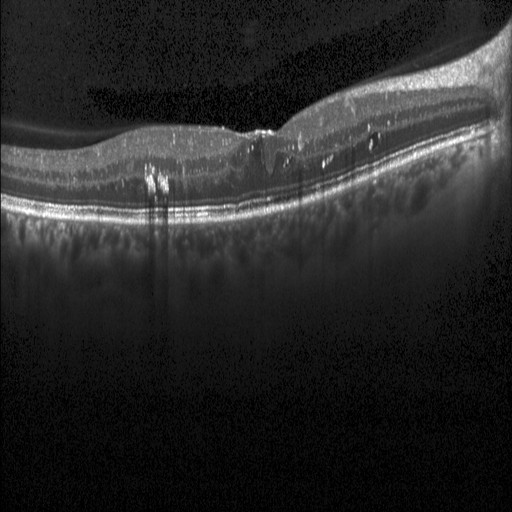

Spectral-domain OCT; OCT B-scan; horizontal scan through the fovea — Macular OCT: diabetic macular edema (DME).